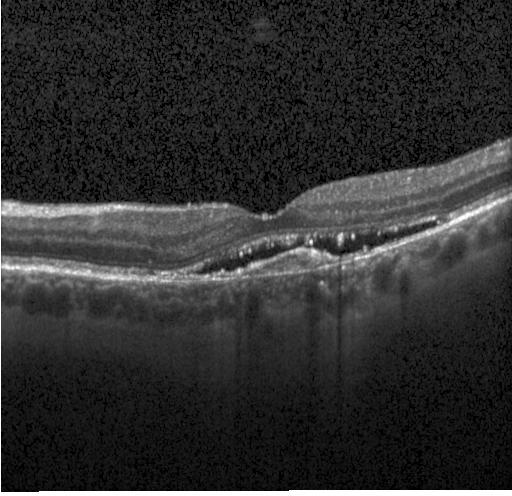

Optical coherence tomography B-scan, spectral-domain optical coherence tomography. Macular OCT: choroidal neovascularization (CNV).